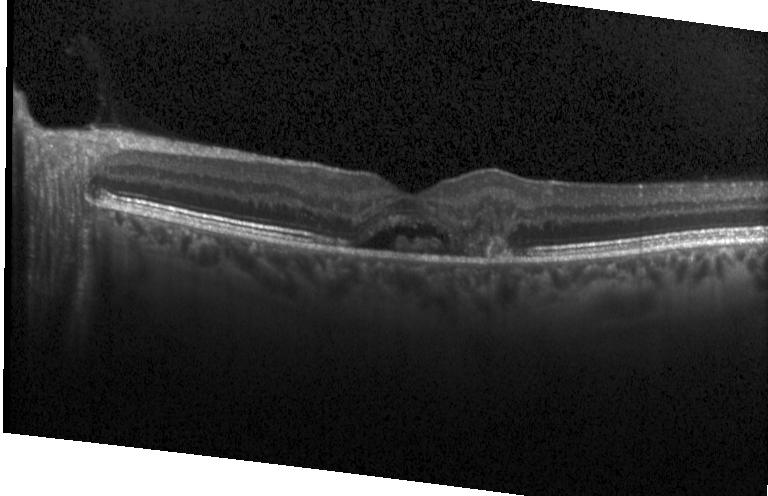
Macular scan, OCT B-scan. The scan shows choroidal neovascularization (CNV).